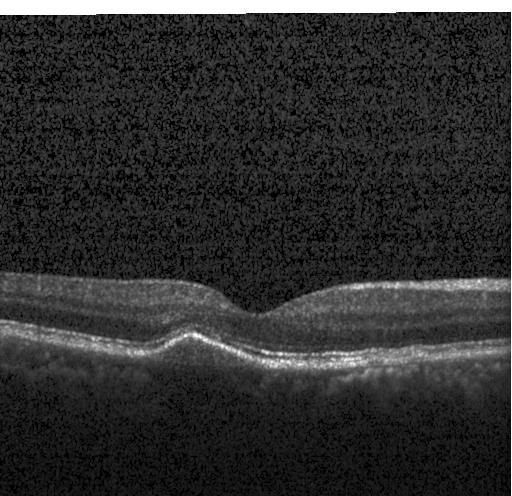
Diagnosis: drusen.